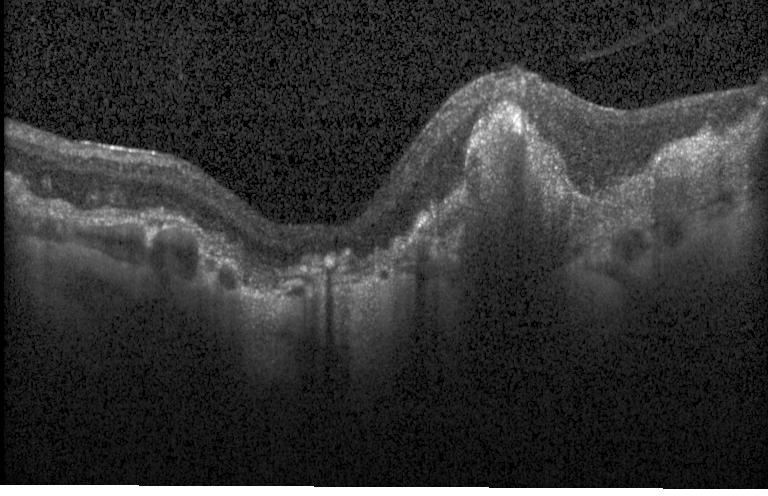 Retinal OCT cross-section · through the macula · spectral-domain OCT
OCT finding: choroidal neovascularization (CNV).